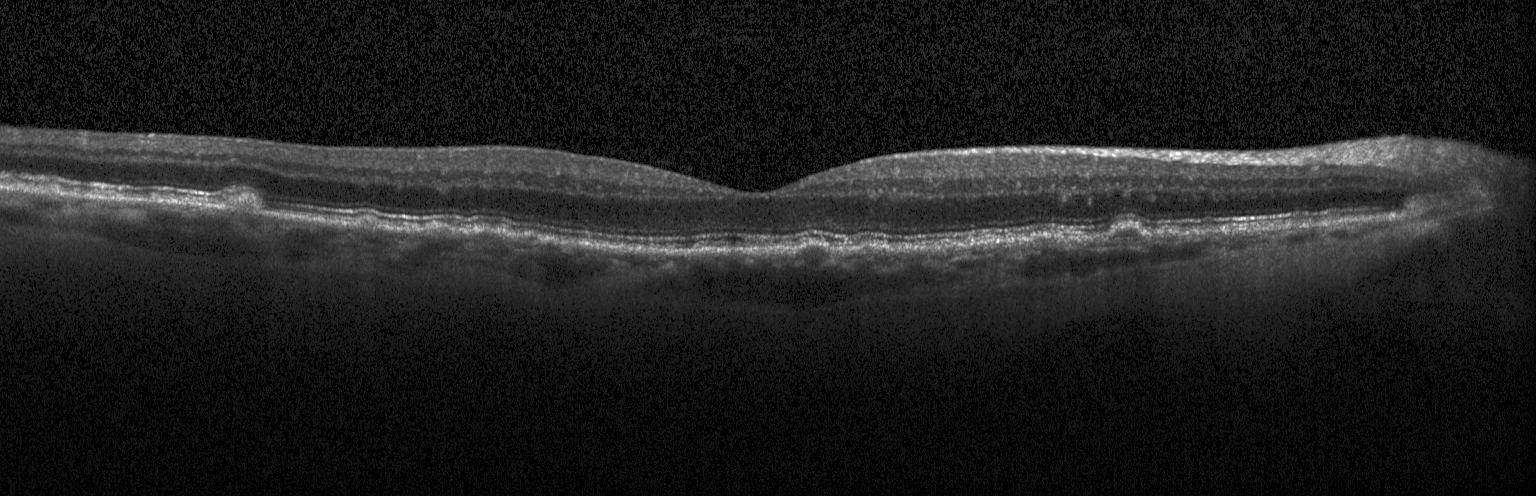 Retinal OCT B-scan. Impression: sub-RPE drusenoid deposits.